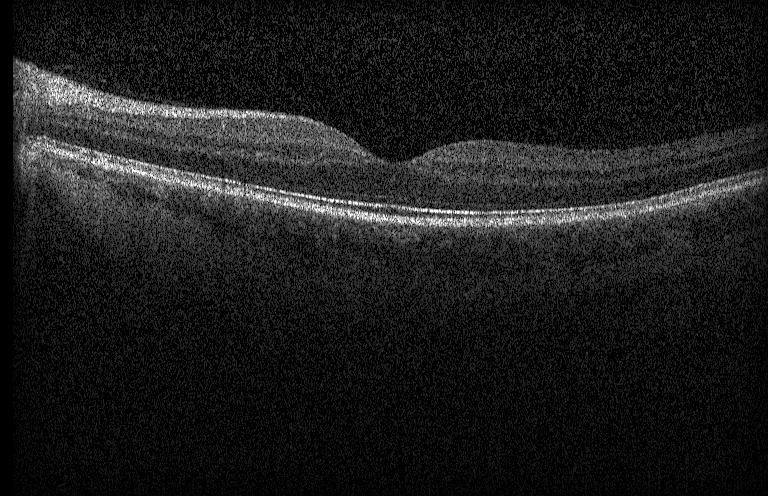

Macular scan. Heidelberg Spectralis. Retinal OCT cross-section. Spectral-domain optical coherence tomography
The scan shows no evidence of CNV, DME, or drusen.